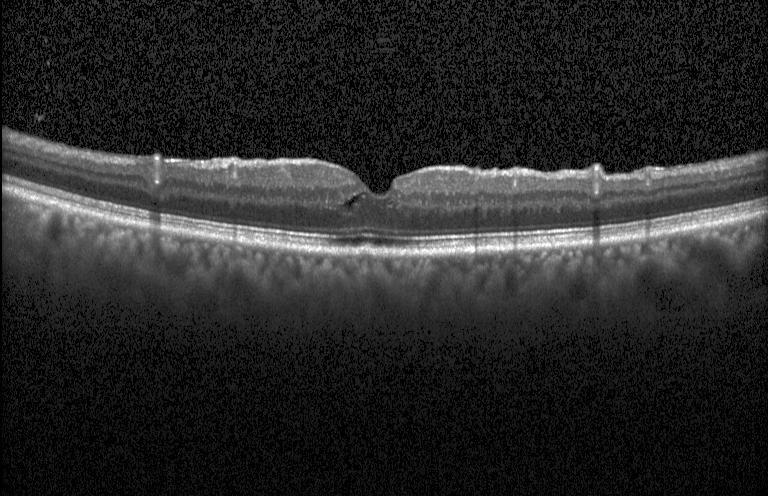 Macular OCT: diabetic macular edema.